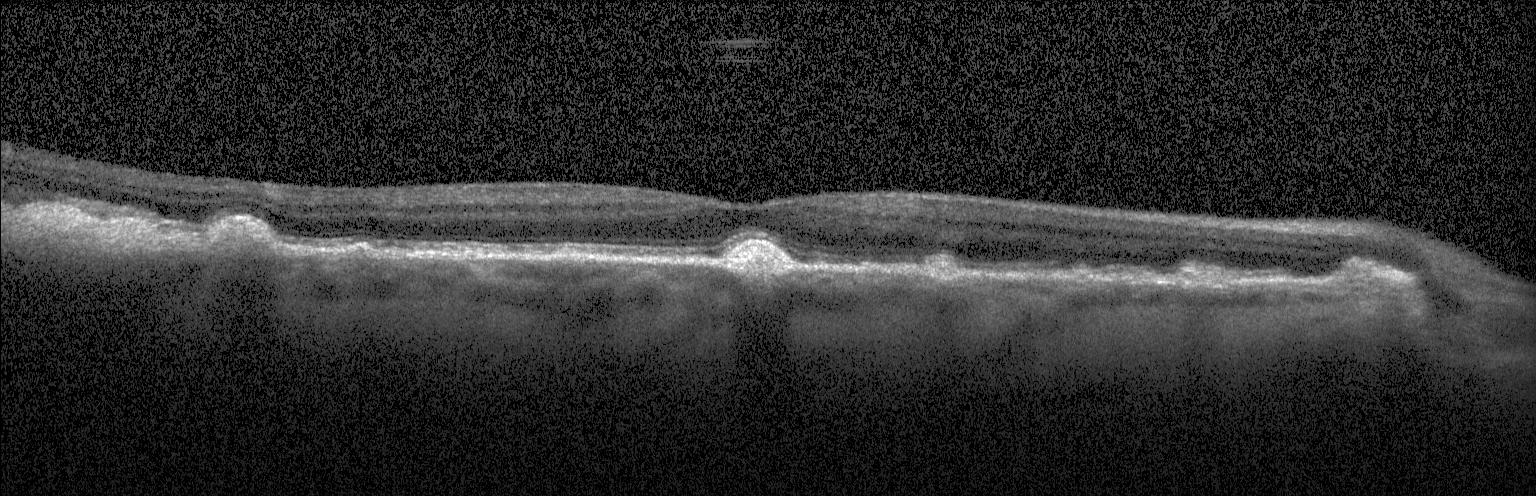
Impression: drusen.